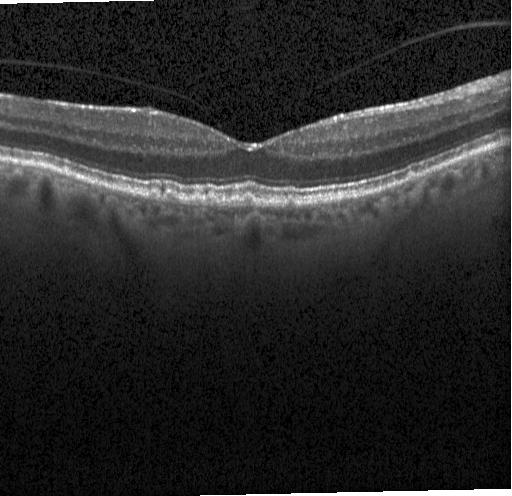

Spectral-domain optical coherence tomography; retinal OCT B-scan
Diagnosis: drusen.